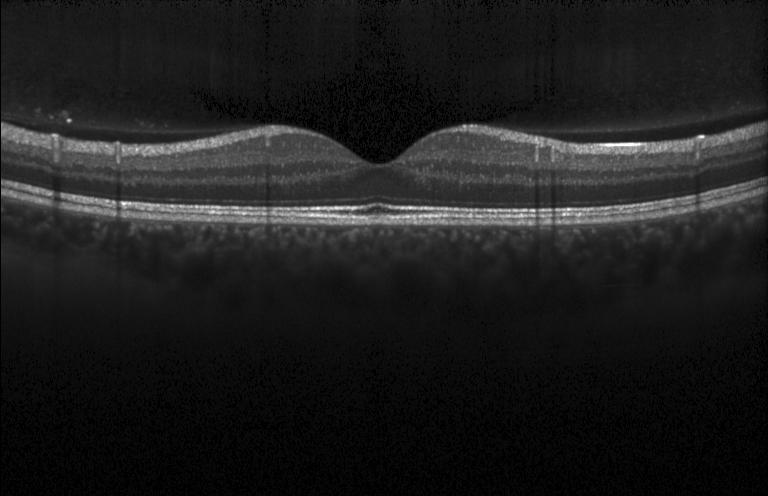 Diagnosis: no evidence of choroidal neovascularization, diabetic macular edema, or drusen.